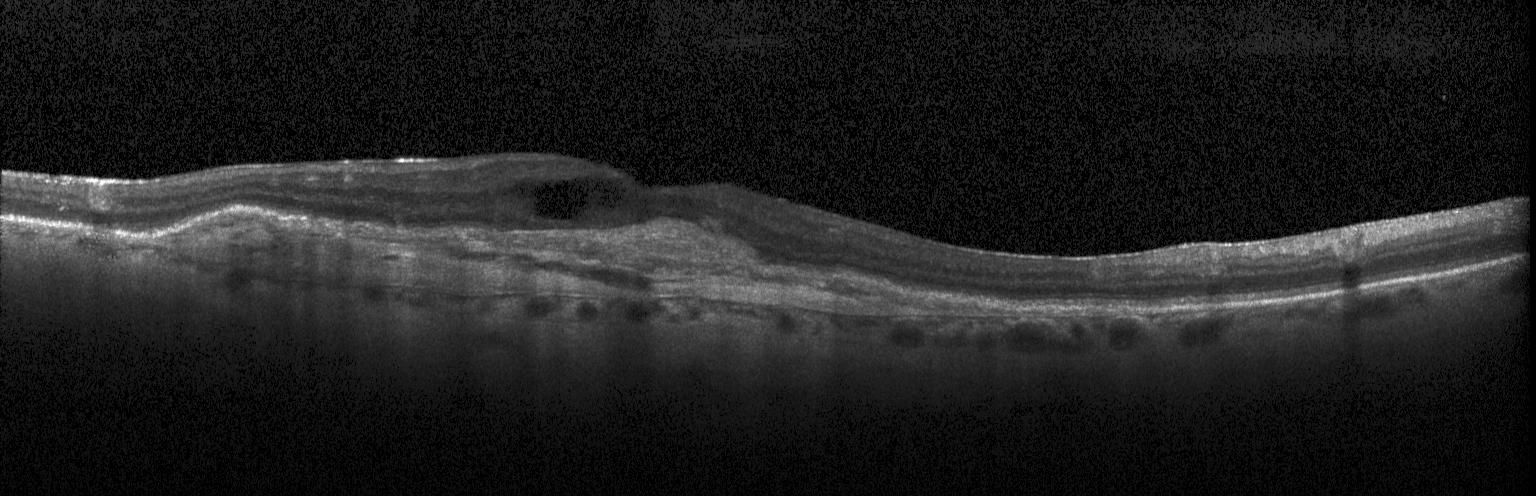

Diagnosis: choroidal neovascularization (CNV).